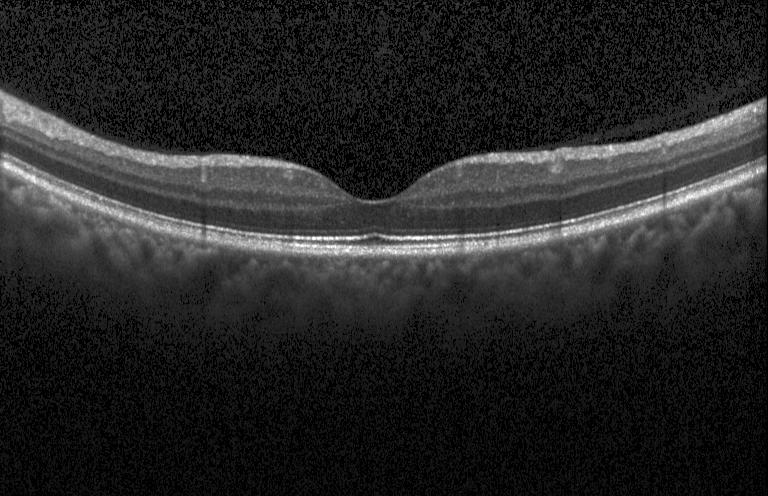

Retinal OCT B-scan, instrument: Heidelberg Spectralis, SD-OCT
Dx: no CNV, DME, or drusen.